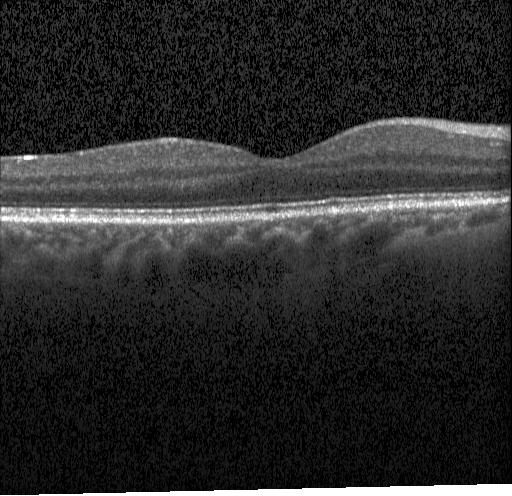

Macular OCT: neither CNV, DME, nor drusen.